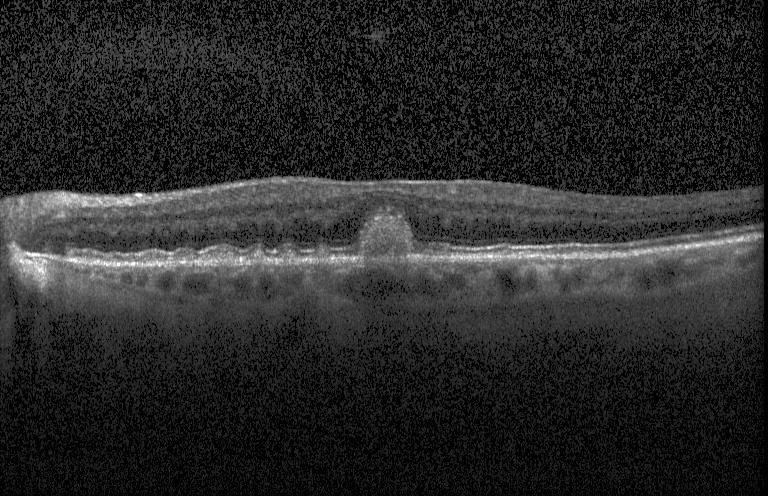
Spectral-domain optical coherence tomography. Retinal OCT cross-section. This B-scan demonstrates choroidal neovascularization.